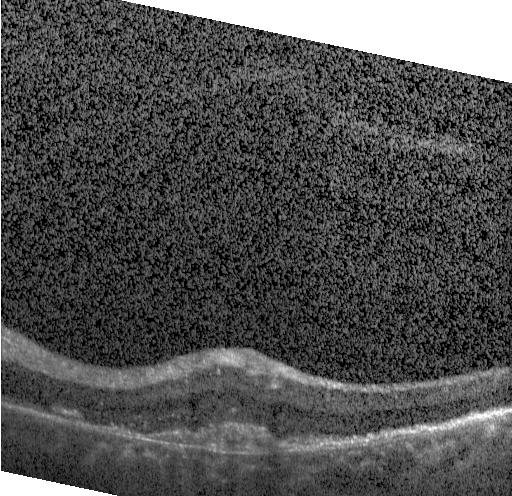 Acquired on a Heidelberg Spectralis · optical coherence tomography scan.
Assessment: choroidal neovascularization.